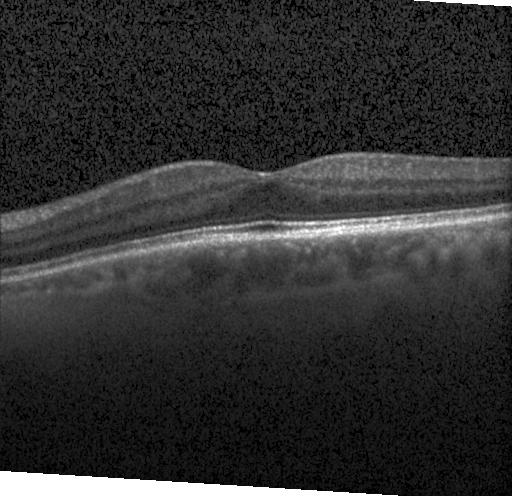
SD-OCT · macular scan · OCT B-scan — Impression: no choroidal neovascularization, diabetic macular edema, or drusen.